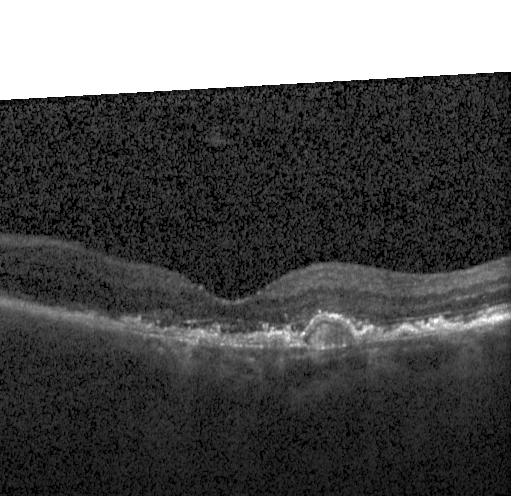
Acquired on a Heidelberg Spectralis · macular scan · OCT B-scan.
Assessment: choroidal neovascularization.